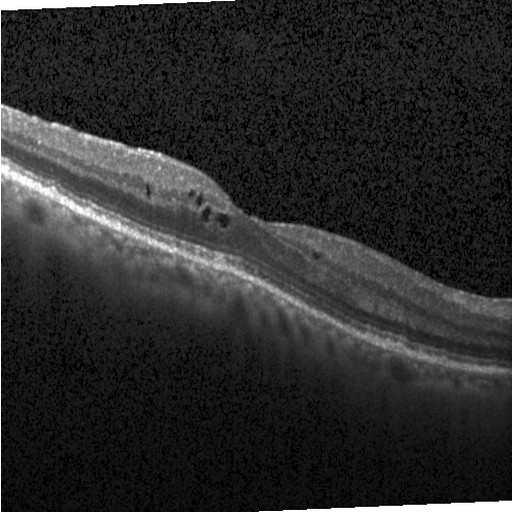
Spectral-domain optical coherence tomography, optical coherence tomography scan, fovea-centered
The scan shows diabetic macular edema (DME).